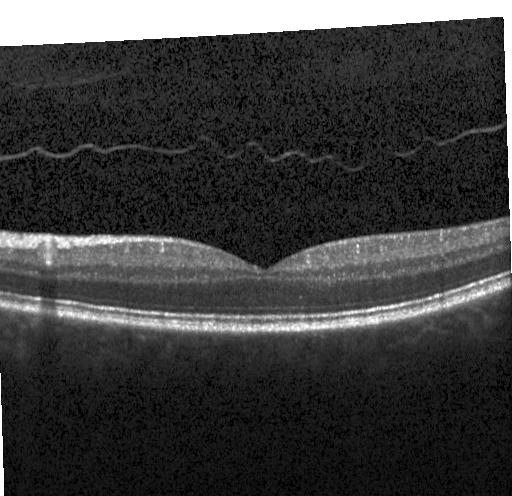

Heidelberg Spectralis; spectral-domain OCT; OCT B-scan.
The scan shows neither choroidal neovascularization, diabetic macular edema, nor drusen.